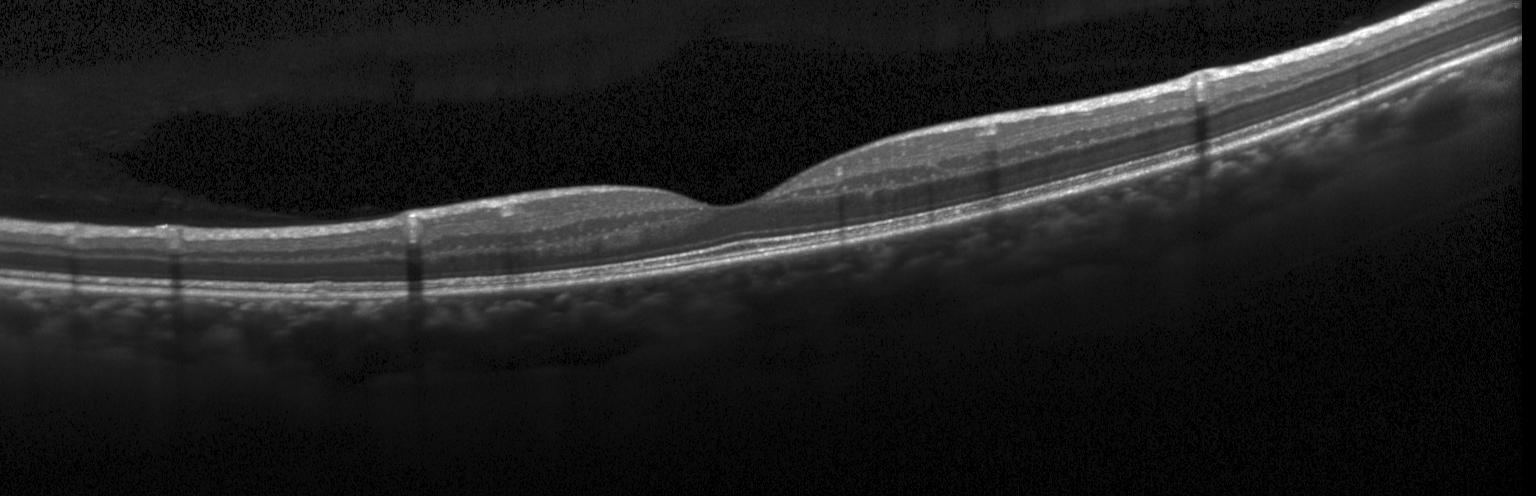 Retinal OCT B-scan, acquired on a Heidelberg Spectralis.
Finding: no CNV, no DME, and no drusen.